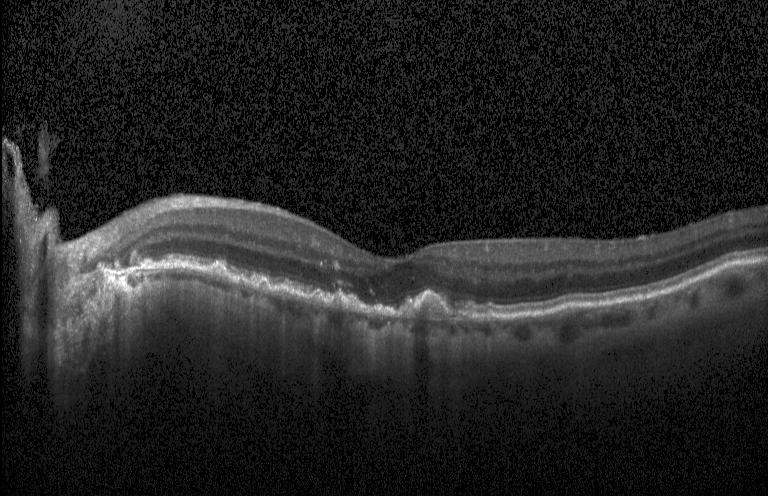 OCT line scan, spectral-domain optical coherence tomography, Heidelberg Spectralis OCT system, macular scan. Multiple drusen.